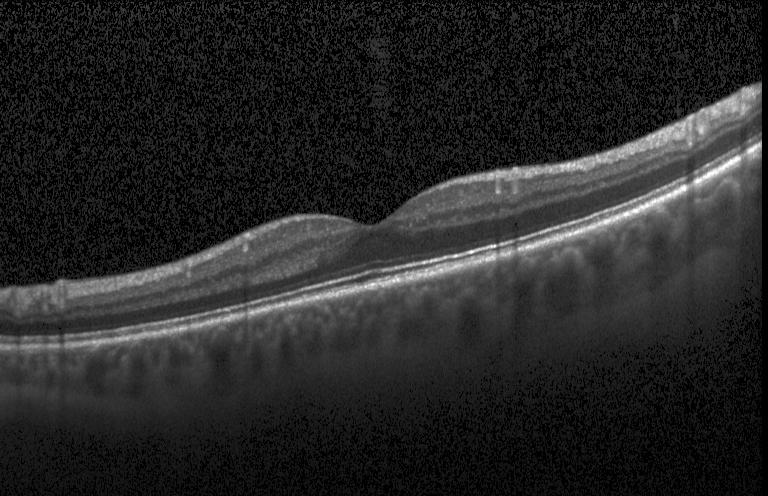 Finding: neither CNV, DME, nor drusen.